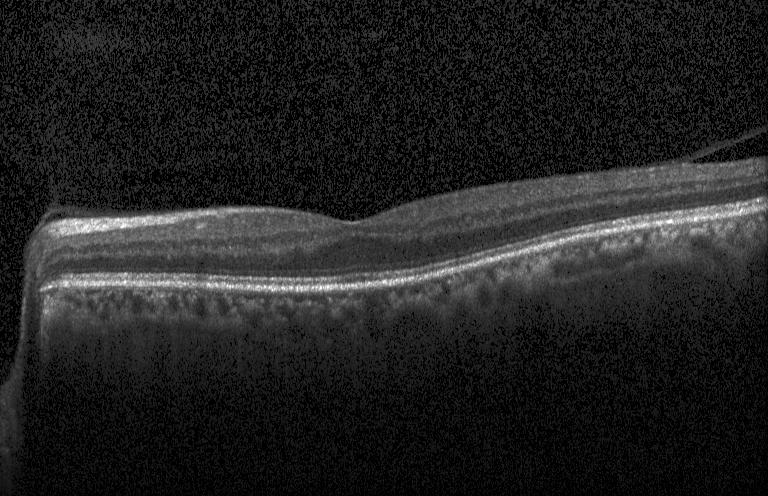 Heidelberg Spectralis · horizontal scan through the fovea · optical coherence tomography scan — Finding: no choroidal neovascularization, diabetic macular edema, or drusen.